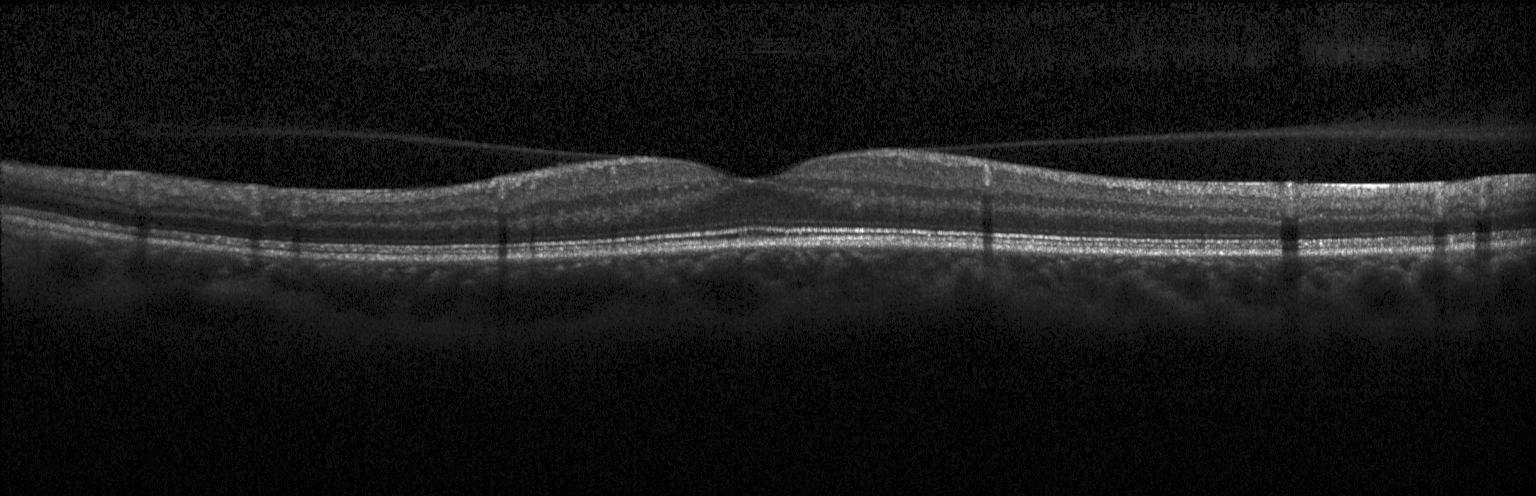 OCT finding: neither choroidal neovascularization, diabetic macular edema, nor drusen.